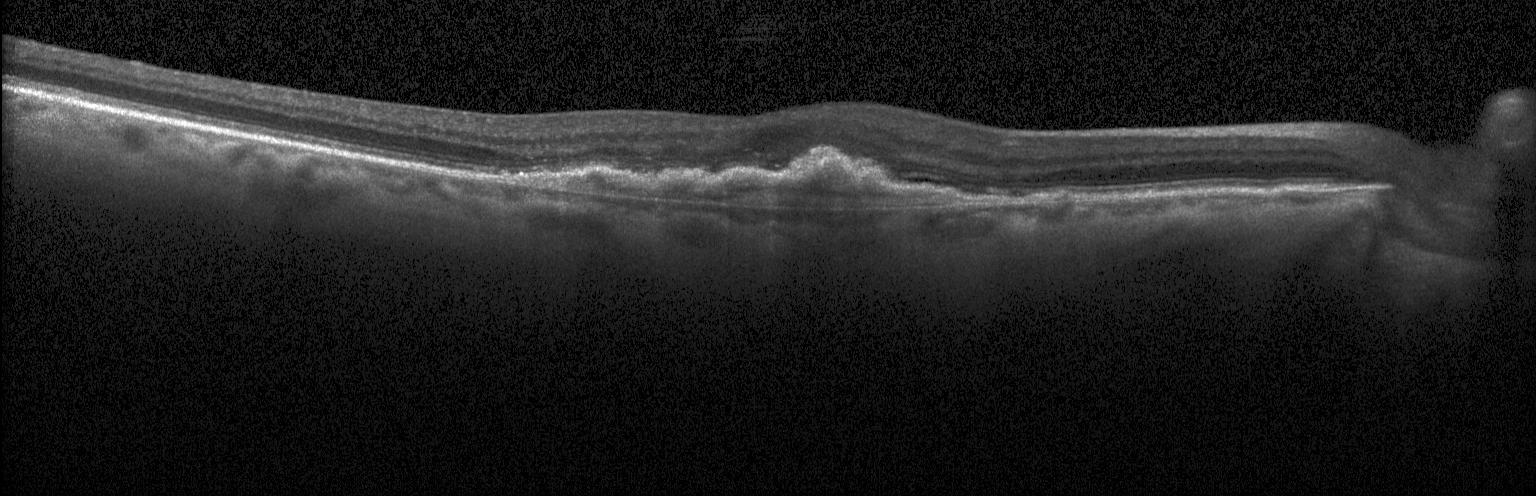
Optical coherence tomography B-scan · spectral-domain OCT · macular scan — The scan shows a choroidal neovascular membrane.